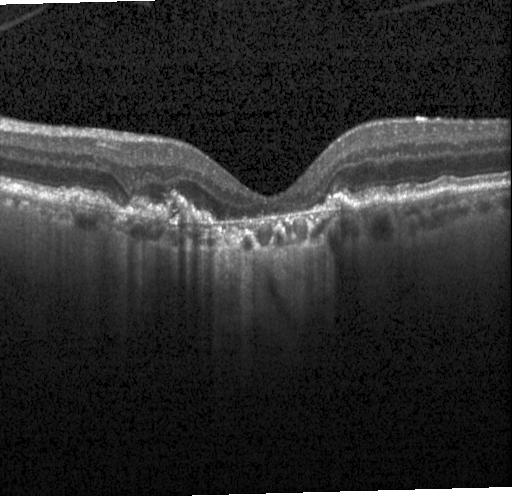 Finding: choroidal neovascularization.